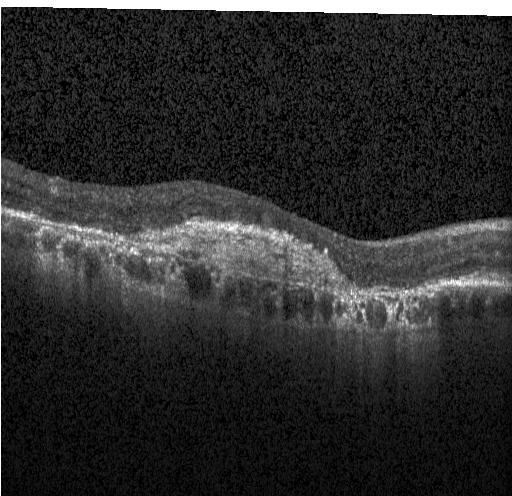
Dx: choroidal neovascularization (CNV).